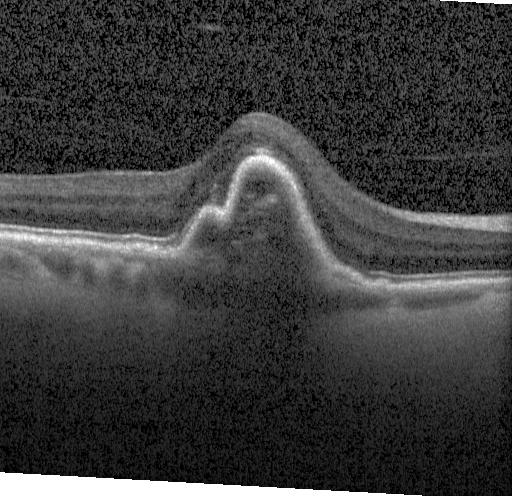 Instrument: Heidelberg Spectralis, retinal OCT B-scan, macular scan — Finding: a choroidal neovascular membrane.